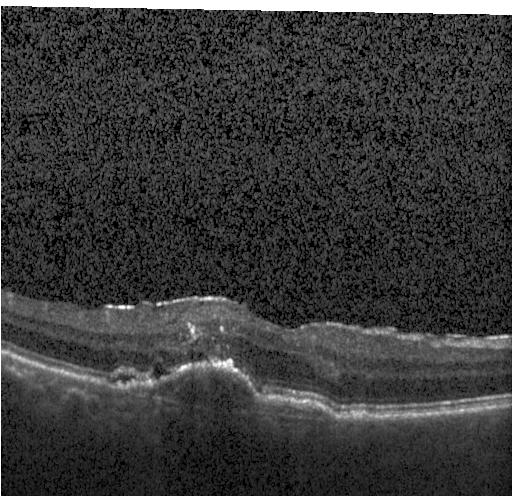
OCT B-scan — Finding: CNV.